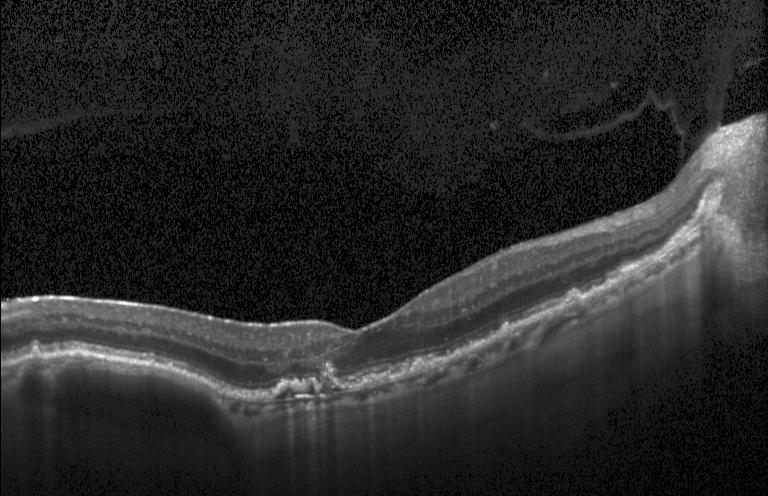
Retinal OCT B-scan. Spectral-domain OCT. Fovea-centered. Heidelberg Spectralis OCT system — Dx: a choroidal neovascular membrane.